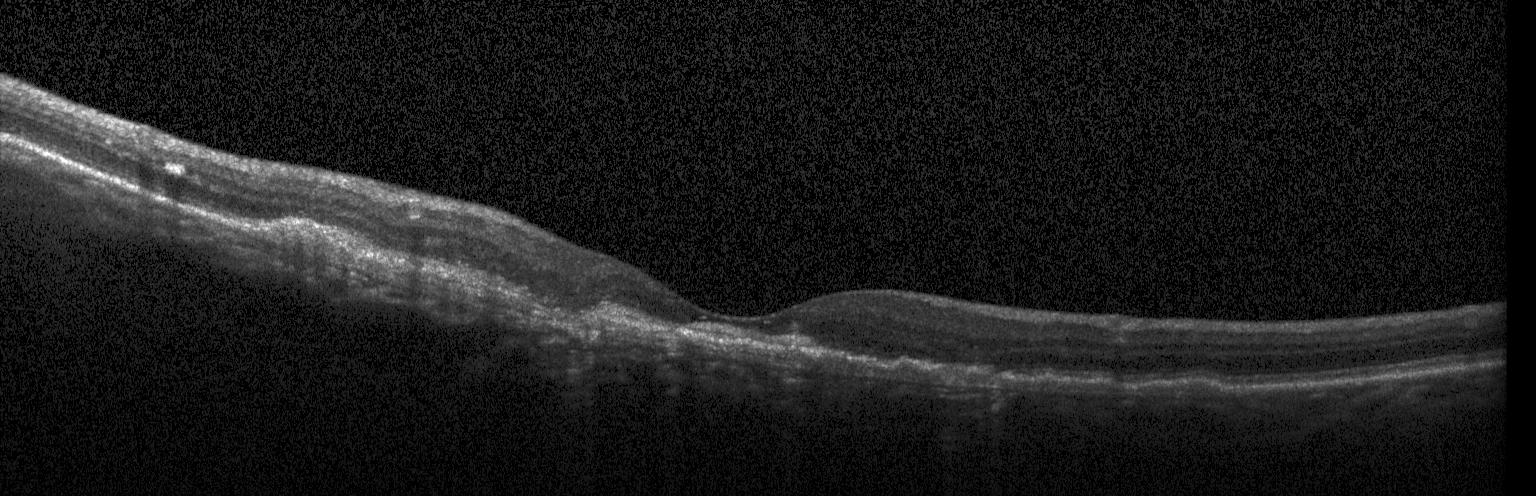
Centered on the fovea. Instrument: Heidelberg Spectralis. Spectral-domain OCT. Optical coherence tomography B-scan.
Finding: a choroidal neovascular membrane.